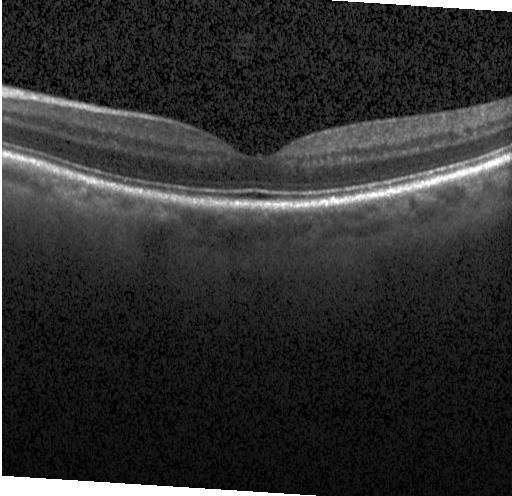
Spectral-domain OCT; retinal OCT cross-section; fovea-centered
Finding: no CNV, no DME, and no drusen.